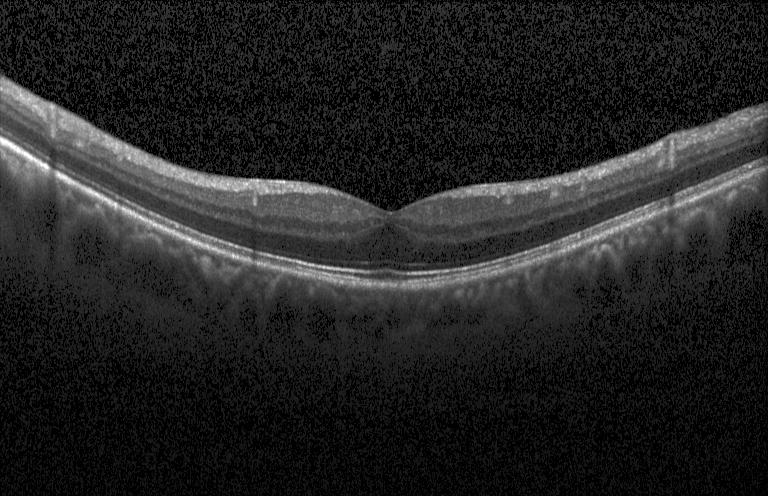
Heidelberg Spectralis. Fovea-centered. Retinal OCT B-scan — Macular OCT: no evidence of choroidal neovascularization, diabetic macular edema, or drusen.